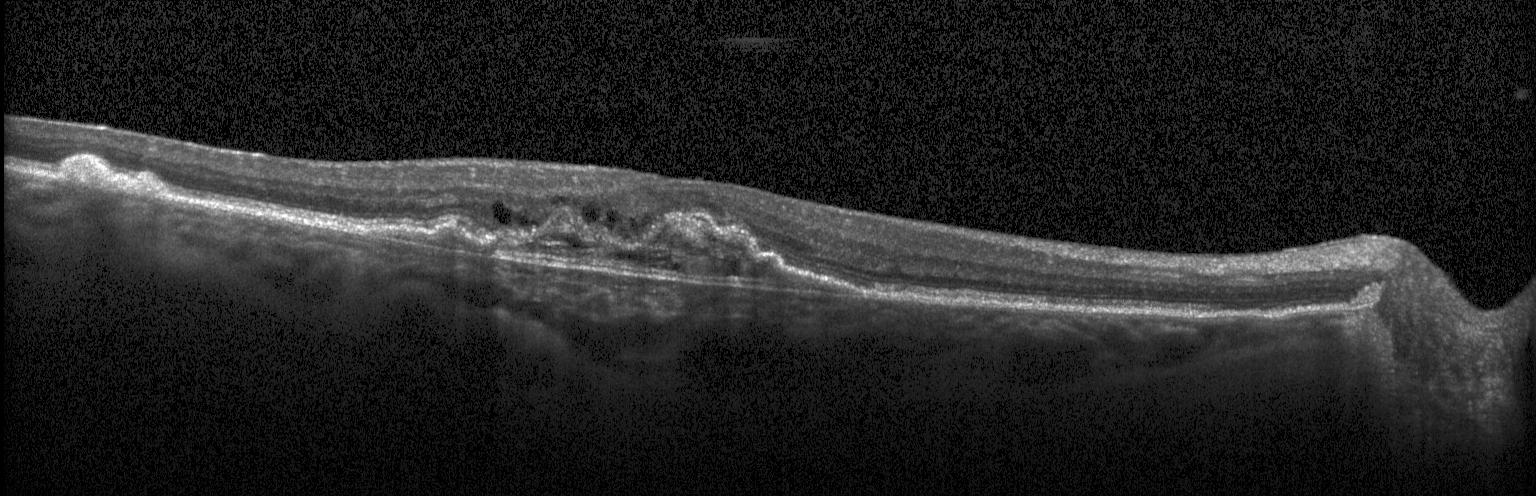 Assessment: a choroidal neovascular membrane.